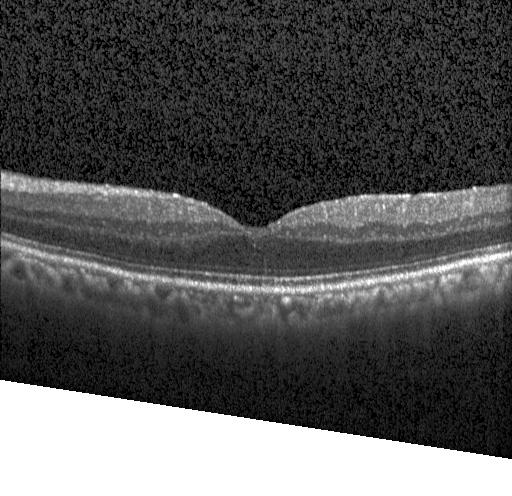 OCT scan showing no choroidal neovascularization, no diabetic macular edema, and no drusen.